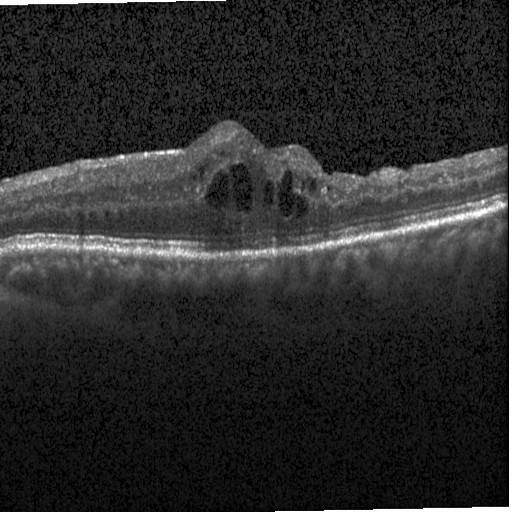

Finding: diabetic macular edema (DME).